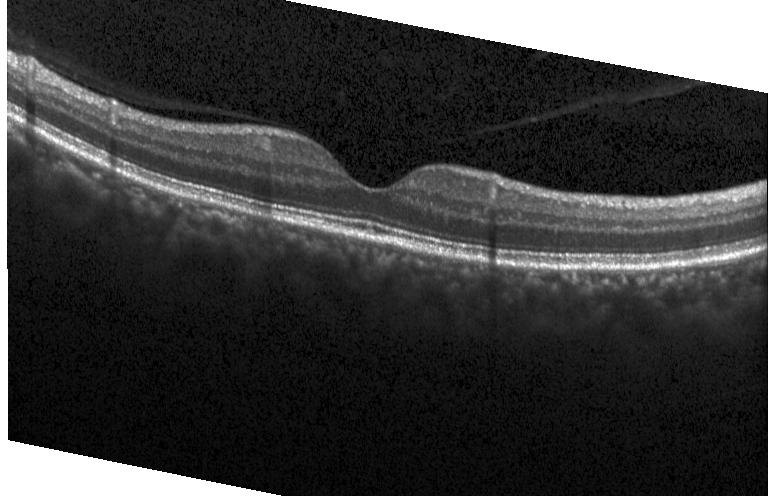

OCT line scan; spectral-domain optical coherence tomography.
Impression: no choroidal neovascularization, diabetic macular edema, or drusen.